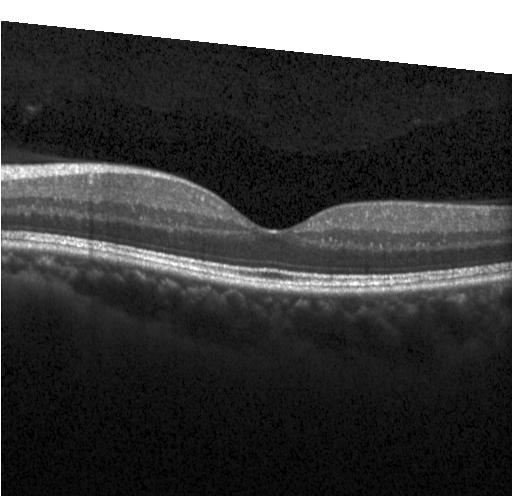 Impression: no choroidal neovascularization, no diabetic macular edema, and no drusen.